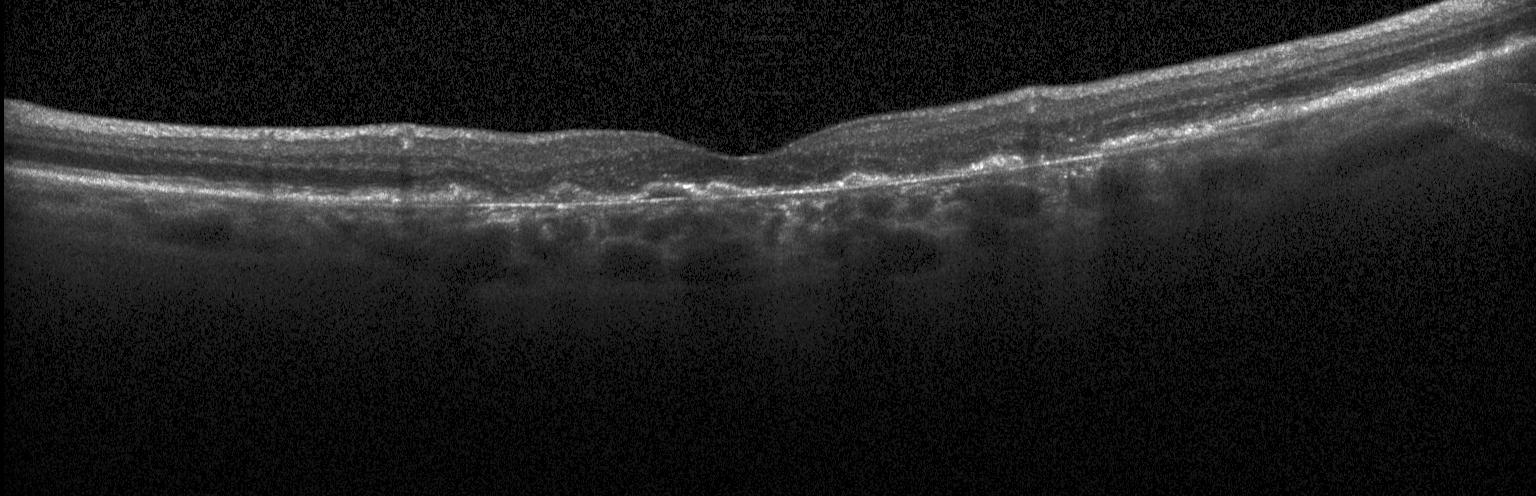 SD-OCT. Optical coherence tomography B-scan. OCT finding: choroidal neovascularization (CNV).